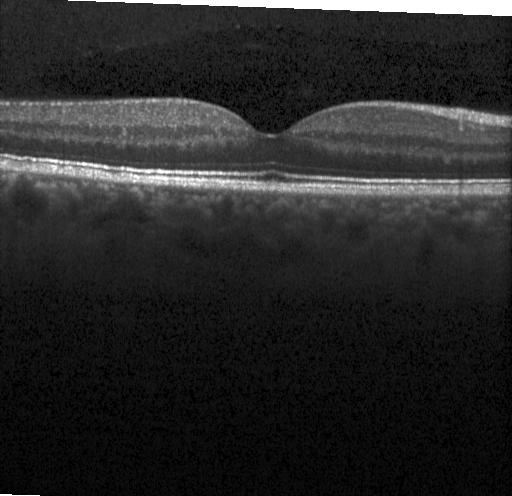
OCT finding: no choroidal neovascularization, no diabetic macular edema, and no drusen.